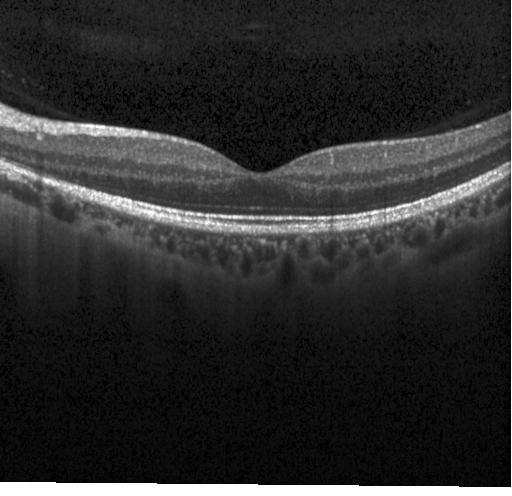 Spectral-domain optical coherence tomography. Optical coherence tomography B-scan. Centered on the fovea
The scan shows no choroidal neovascularization, diabetic macular edema, or drusen.